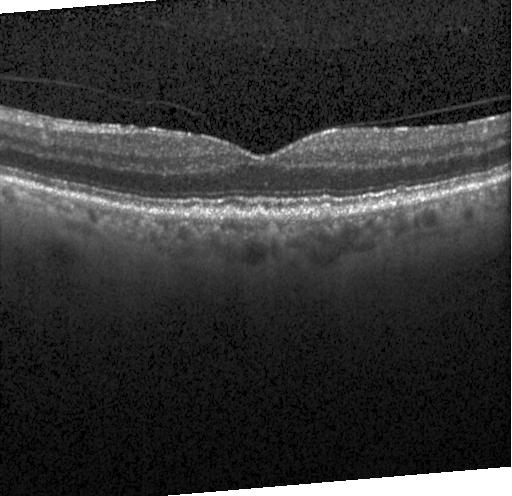 Optical coherence tomography B-scan, spectral-domain OCT, centered on the fovea, instrument: Heidelberg Spectralis — Assessment: sub-RPE drusenoid deposits.